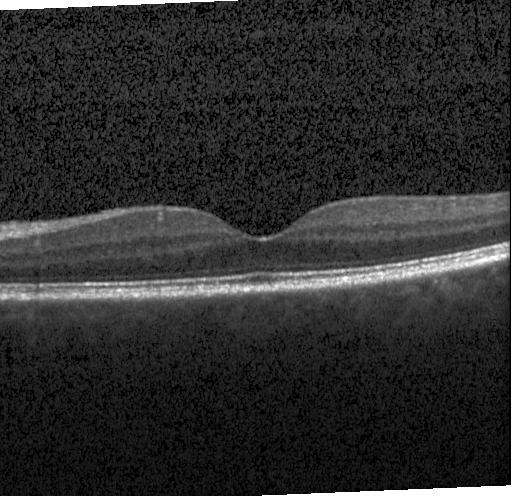
OCT line scan, Heidelberg Spectralis OCT system, spectral-domain optical coherence tomography
The scan shows no evidence of CNV, DME, or drusen.